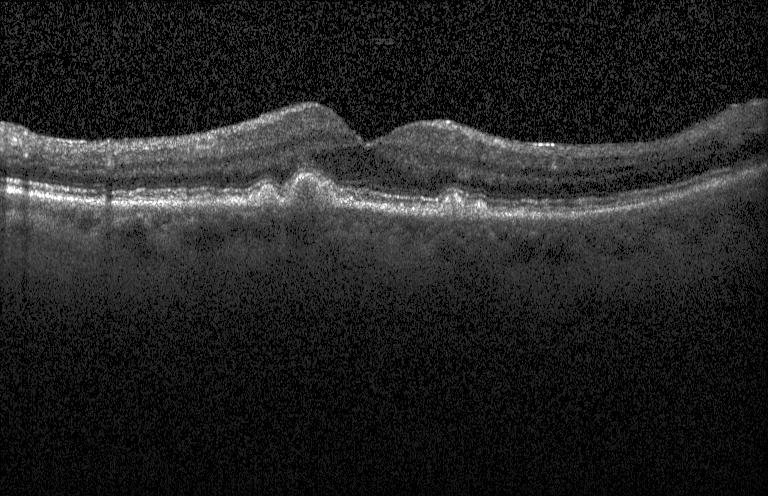 Impression: drusen.